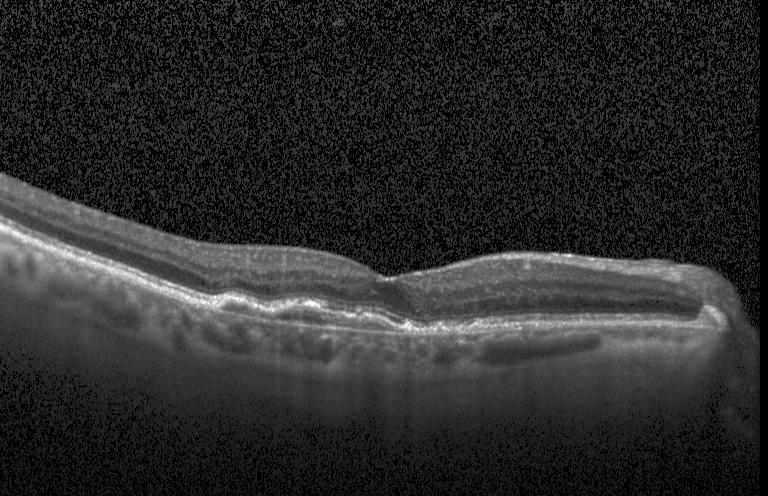

Finding: a choroidal neovascular membrane.